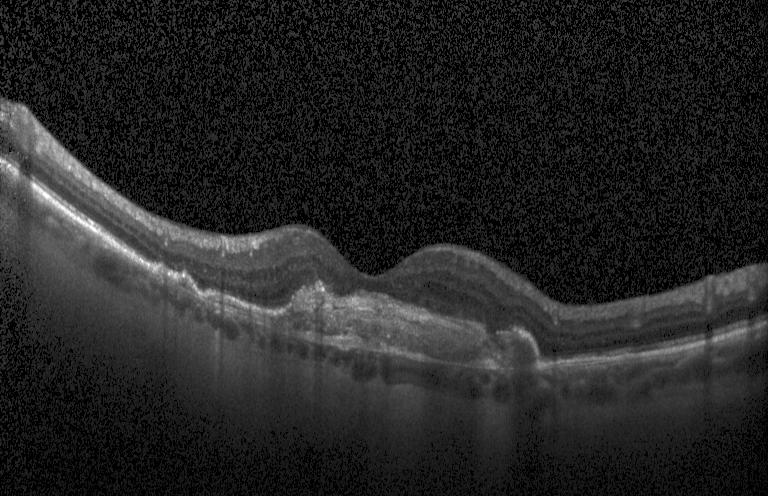
Spectral-domain optical coherence tomography, OCT B-scan
Diagnosis: a choroidal neovascular membrane.